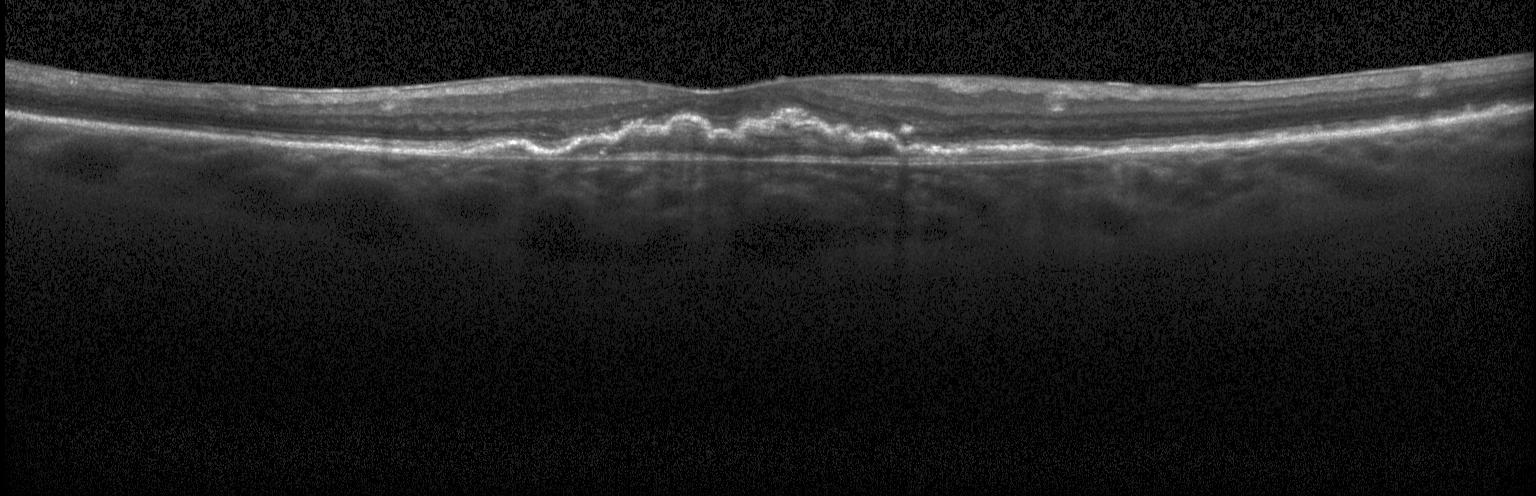

Diagnosis: a choroidal neovascular membrane.